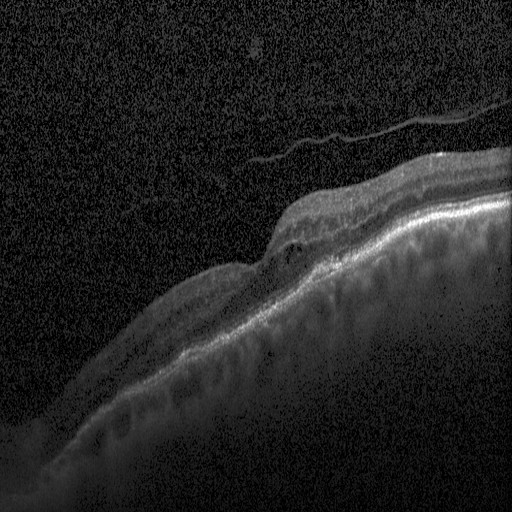 Retinal OCT B-scan.
Impression: diabetic macular edema (DME).